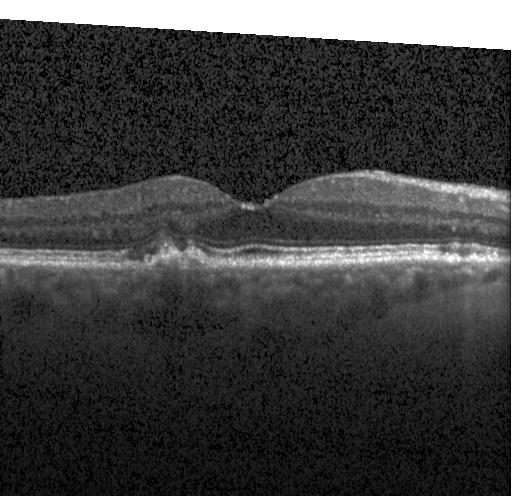

Optical coherence tomography B-scan · Heidelberg Spectralis OCT system · centered on the fovea · spectral-domain optical coherence tomography
Dx: a choroidal neovascular membrane.